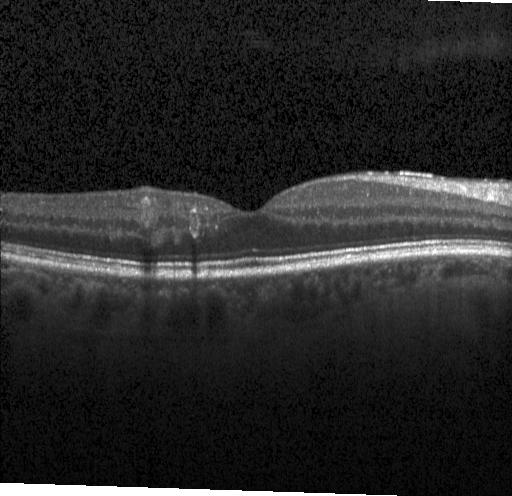 Diagnosis: neither choroidal neovascularization, diabetic macular edema, nor drusen.